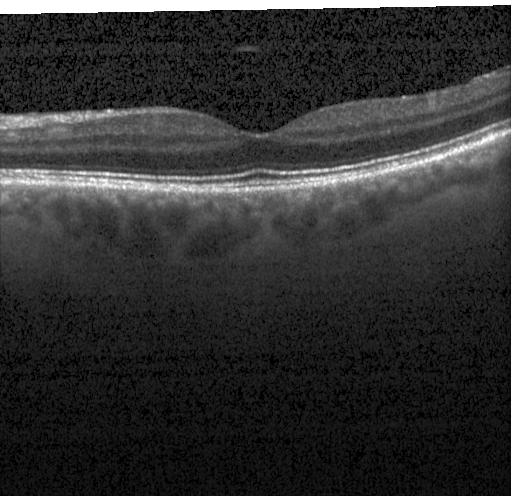
Fovea-centered, Heidelberg Spectralis OCT system, optical coherence tomography scan.
Diagnosis: no choroidal neovascularization, no diabetic macular edema, and no drusen.